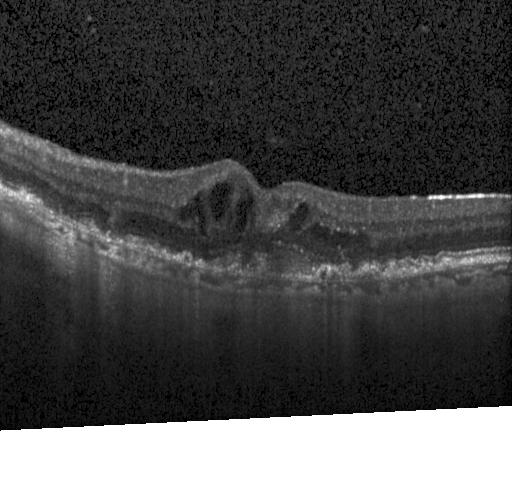

SD-OCT · retinal OCT B-scan · instrument: Heidelberg Spectralis · fovea-centered.
The scan shows choroidal neovascularization.